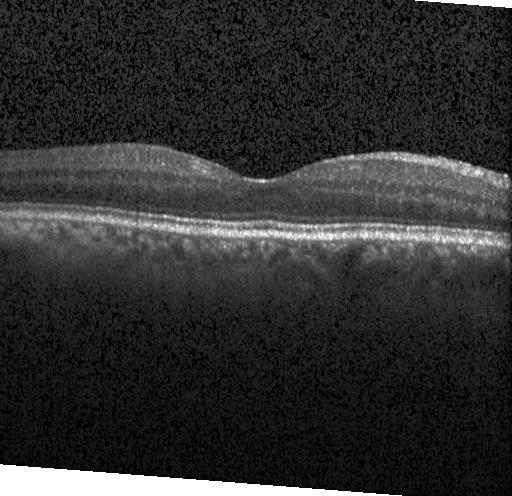

Fovea-centered, OCT B-scan, Heidelberg Spectralis. OCT finding: no evidence of CNV, DME, or drusen.